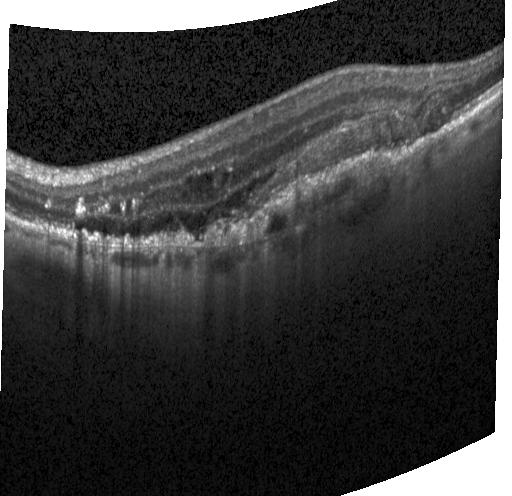

SD-OCT; macular scan; optical coherence tomography scan.
Dx: a choroidal neovascular membrane.